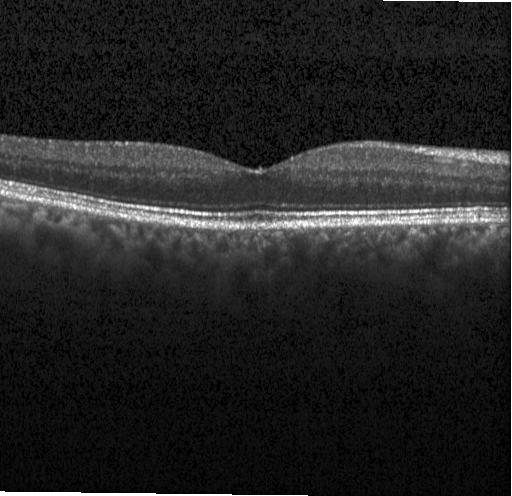
SD-OCT · OCT B-scan — Dx: no choroidal neovascularization, diabetic macular edema, or drusen.